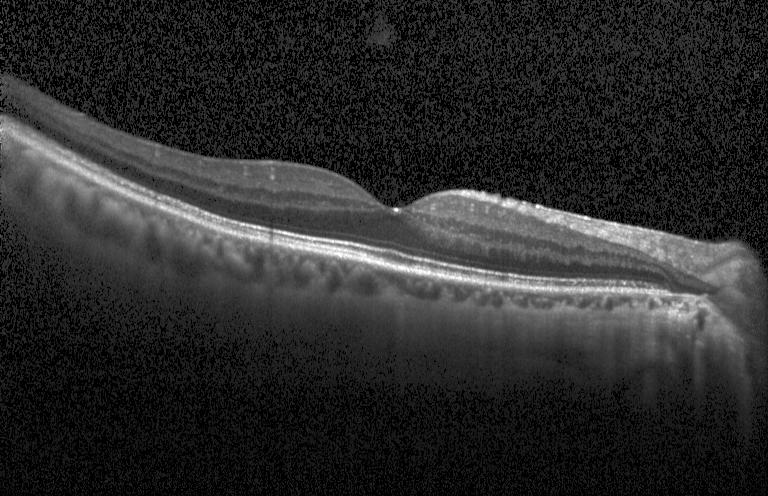

Optical coherence tomography B-scan · Heidelberg Spectralis.
Impression: no evidence of CNV, DME, or drusen.